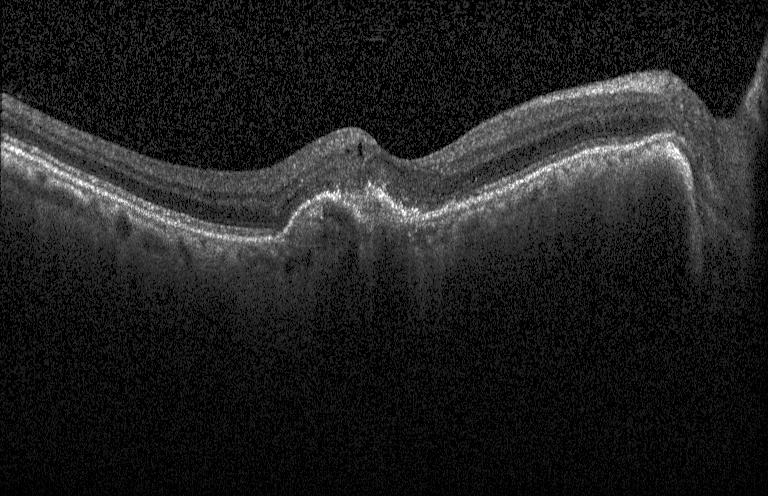
Macular OCT demonstrating choroidal neovascularization (CNV).